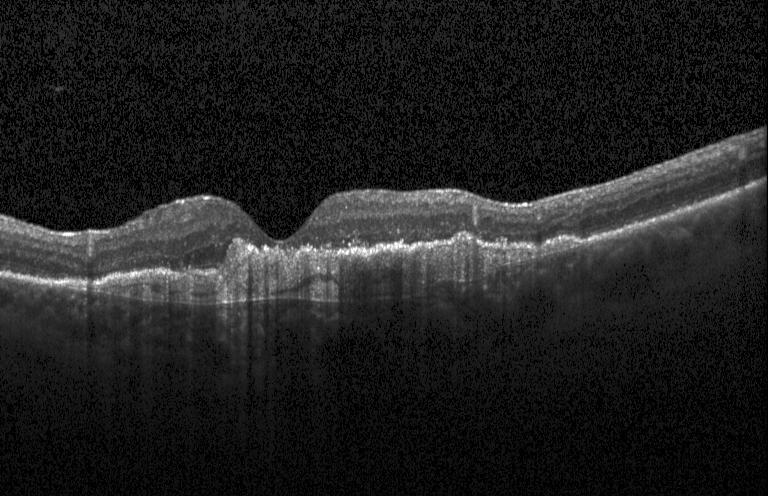
Macular scan; spectral-domain OCT; optical coherence tomography B-scan; Heidelberg Spectralis
A choroidal neovascular membrane.